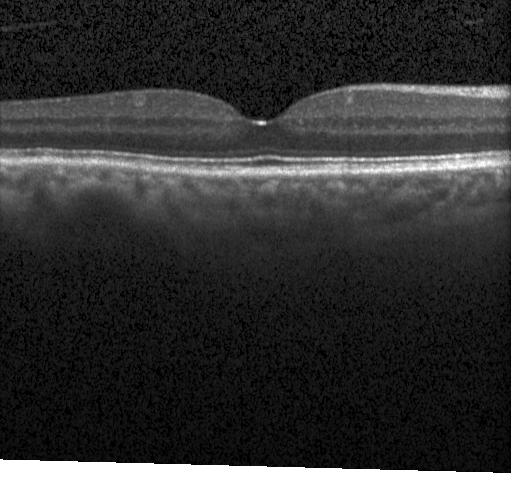

Macular OCT: neither choroidal neovascularization, diabetic macular edema, nor drusen.